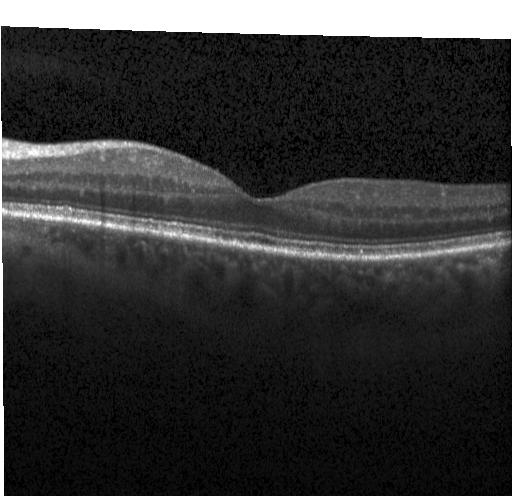
Acquired on a Heidelberg Spectralis · optical coherence tomography B-scan · centered on the fovea
The scan shows no choroidal neovascularization, no diabetic macular edema, and no drusen.